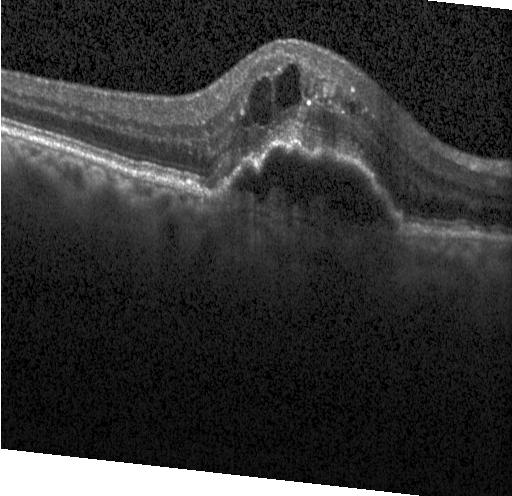
OCT finding: a choroidal neovascular membrane.